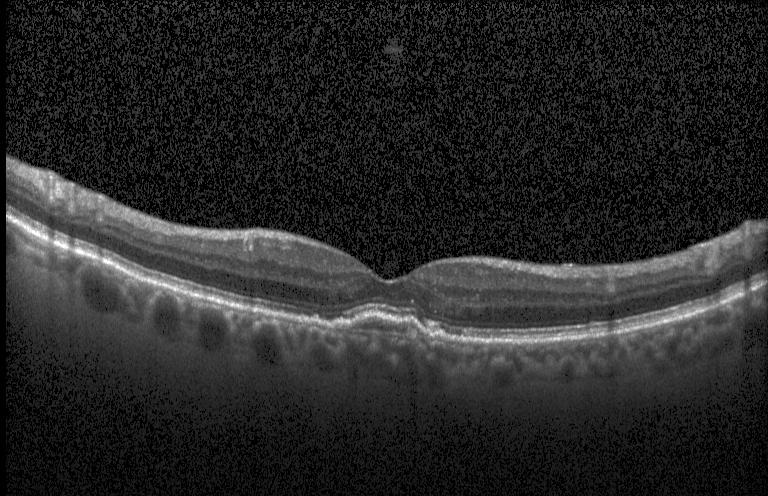

OCT line scan.
A choroidal neovascular membrane.